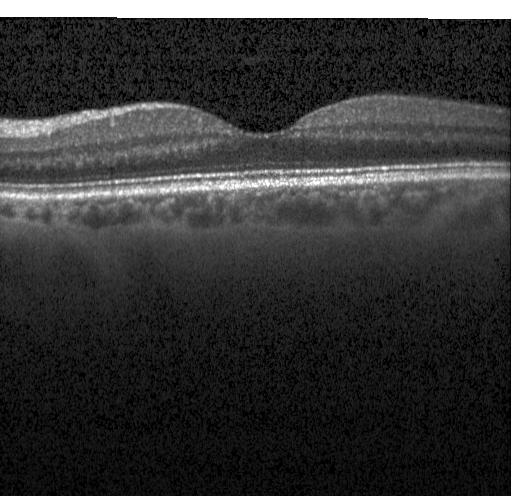
SD-OCT · optical coherence tomography scan · acquired on a Heidelberg Spectralis · macular scan
This B-scan demonstrates no CNV, no DME, and no drusen.